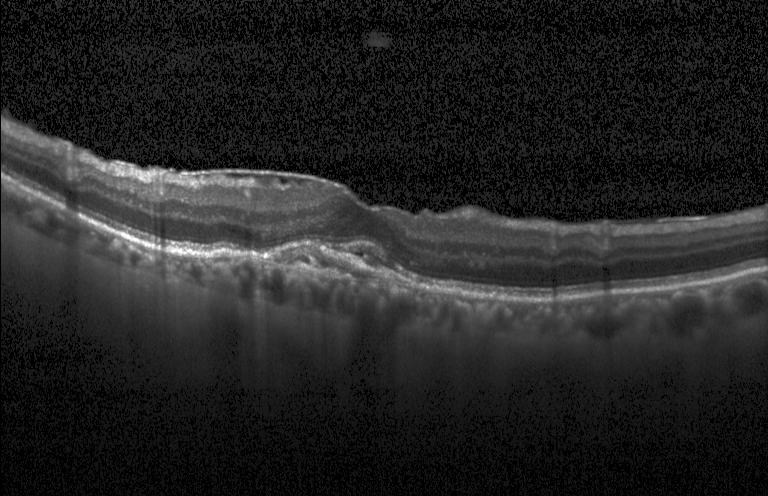

OCT finding: choroidal neovascularization.